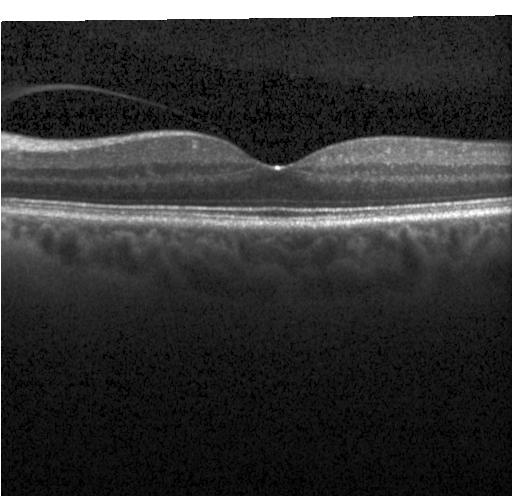 Retinal OCT B-scan. Diagnosis: no evidence of choroidal neovascularization, diabetic macular edema, or drusen.